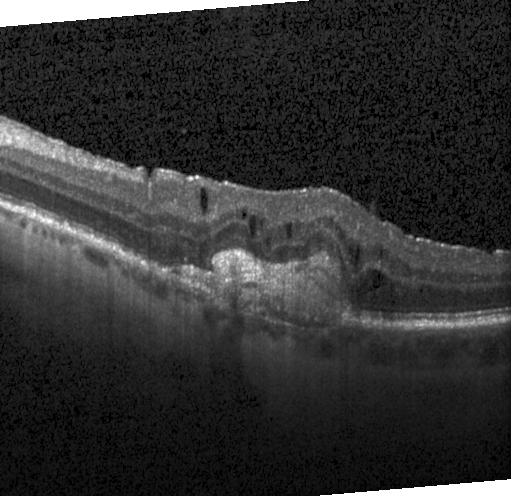 Heidelberg Spectralis · fovea-centered · retinal OCT B-scan. Dx: choroidal neovascularization.